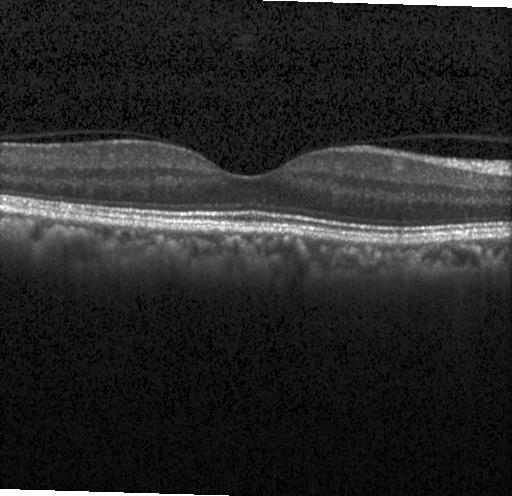
Through the macula. Heidelberg Spectralis. Retinal OCT cross-section — Impression: no choroidal neovascularization, no diabetic macular edema, and no drusen.